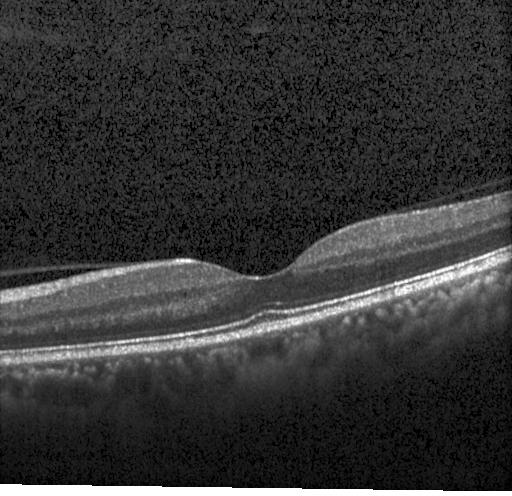
Fovea-centered, instrument: Heidelberg Spectralis, retinal OCT B-scan, spectral-domain OCT. Finding: no choroidal neovascularization, diabetic macular edema, or drusen.